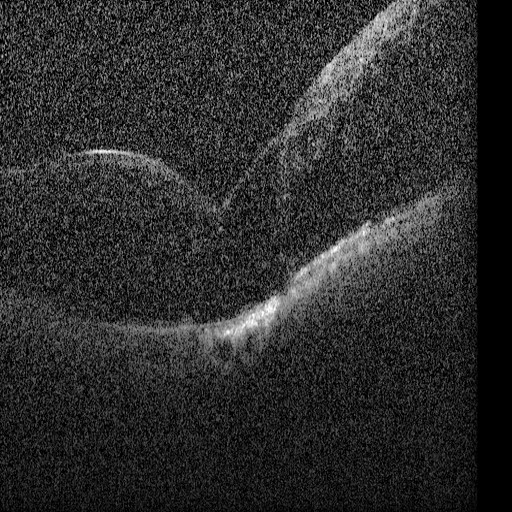 OCT line scan.
Dx: diabetic macular edema (DME).